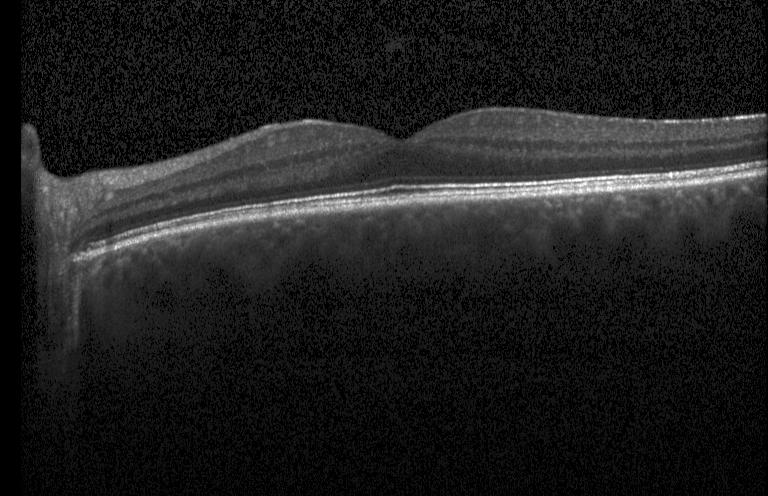
Heidelberg Spectralis OCT system. Centered on the fovea. OCT B-scan. Spectral-domain optical coherence tomography. Impression: no CNV, no DME, and no drusen.